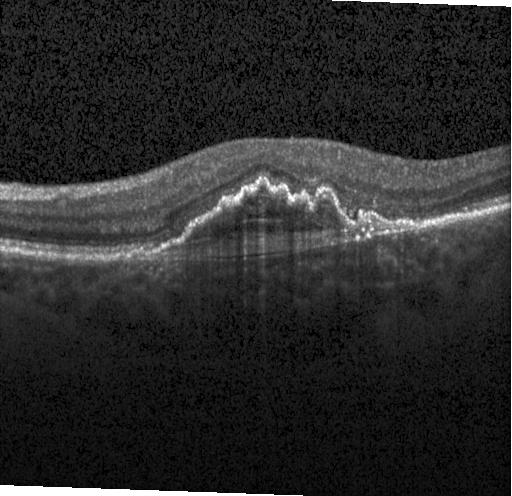

Spectral-domain OCT B-scan: CNV.